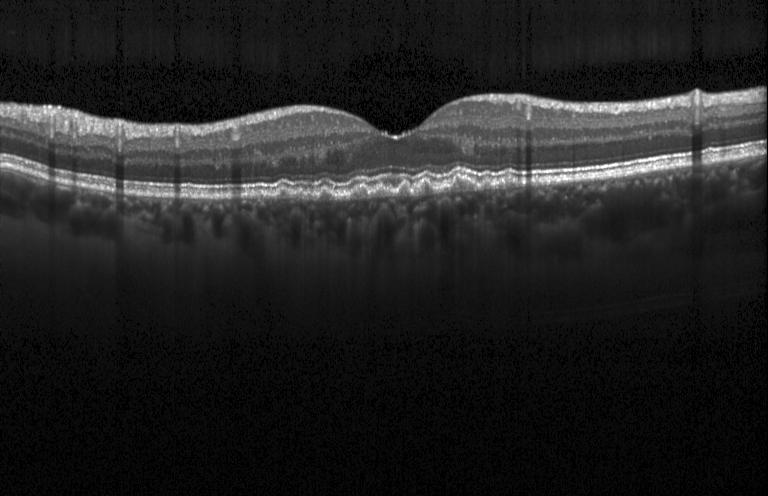
Spectral-domain OCT; retinal OCT B-scan — The scan shows multiple drusen.